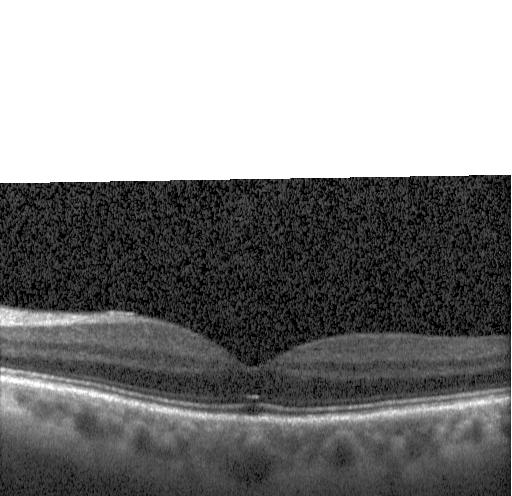 Optical coherence tomography B-scan — Diagnosis: no CNV, DME, or drusen.